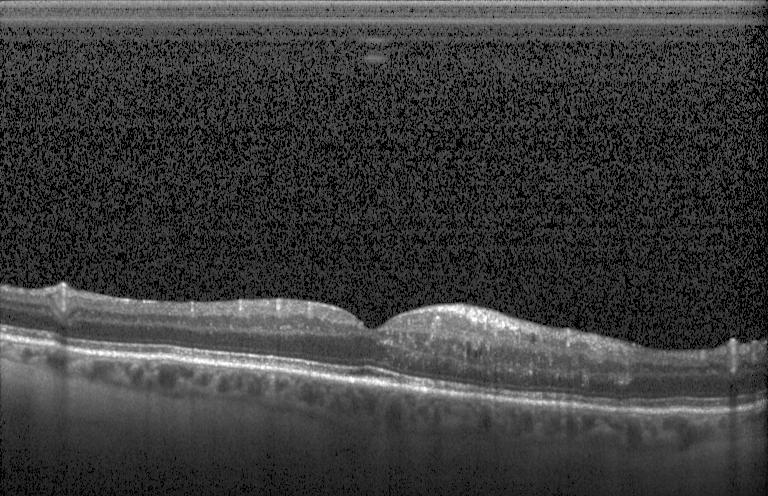 Diagnosis: diabetic macular edema (DME).